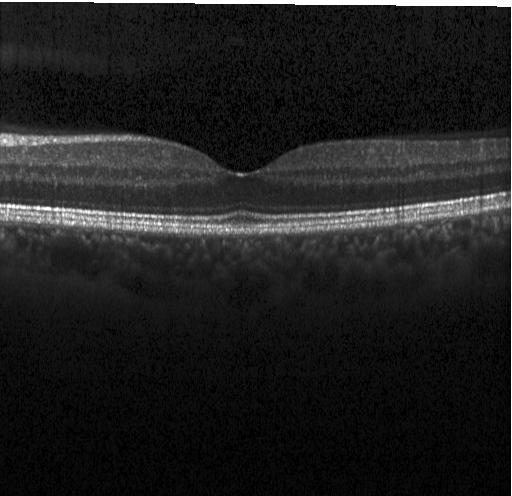 Impression: no evidence of CNV, DME, or drusen.